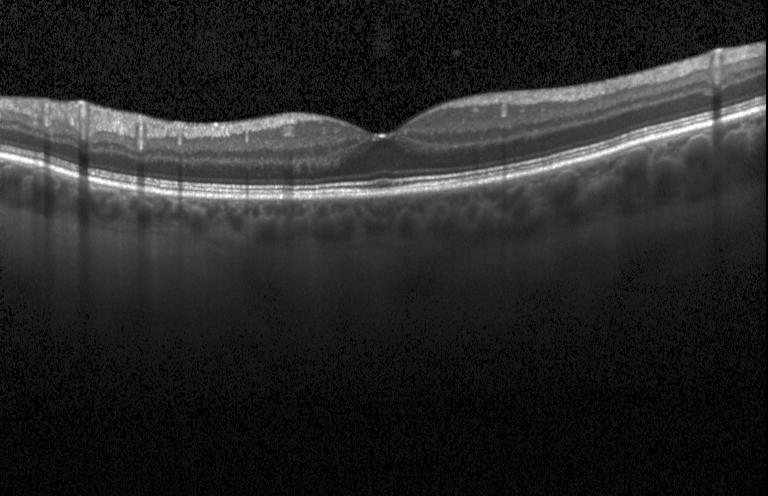
Horizontal scan through the fovea; retinal OCT B-scan
No choroidal neovascularization, no diabetic macular edema, and no drusen.